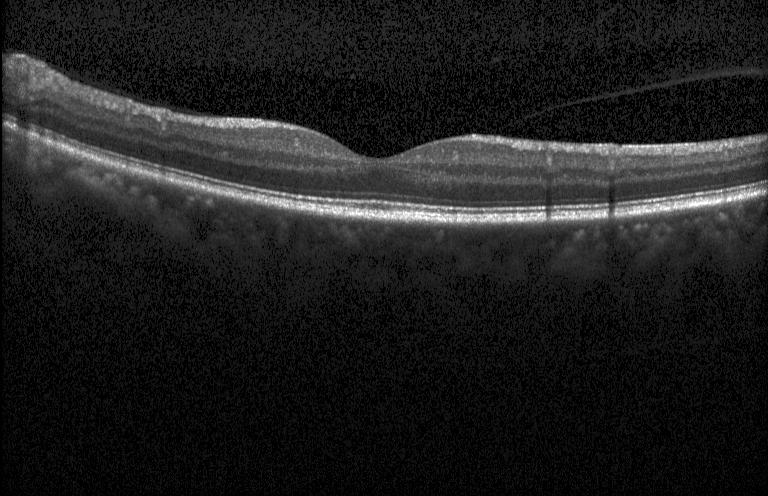
Instrument: Heidelberg Spectralis. Retinal OCT cross-section
Macular OCT: no evidence of choroidal neovascularization, diabetic macular edema, or drusen.